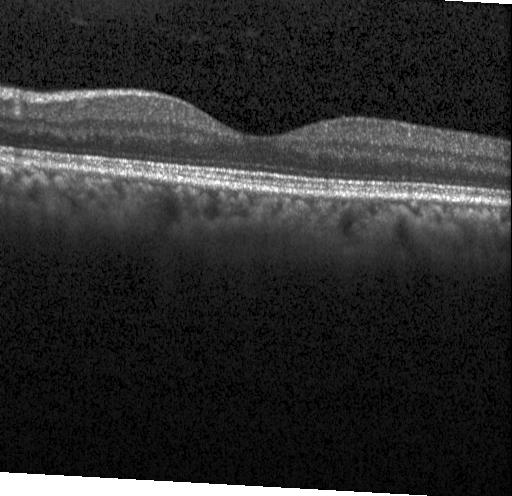

Optical coherence tomography B-scan, fovea-centered. Dx: no choroidal neovascularization, diabetic macular edema, or drusen.